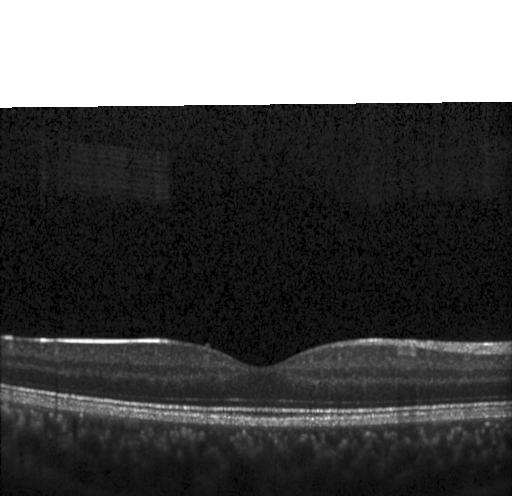
Instrument: Heidelberg Spectralis. Fovea-centered. SD-OCT. OCT line scan. Macular OCT: no evidence of CNV, DME, or drusen.